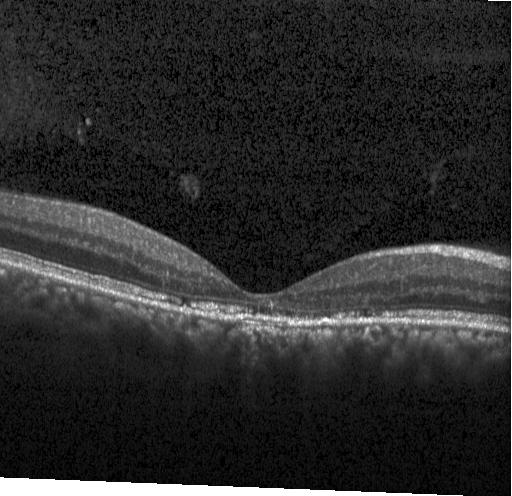
Retinal OCT B-scan. Centered on the fovea. Heidelberg Spectralis. Impression: CNV.